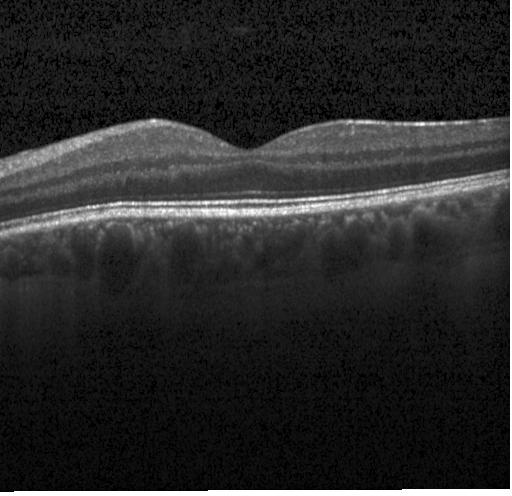 Acquired on a Heidelberg Spectralis · retinal OCT B-scan.
Neither choroidal neovascularization, diabetic macular edema, nor drusen.